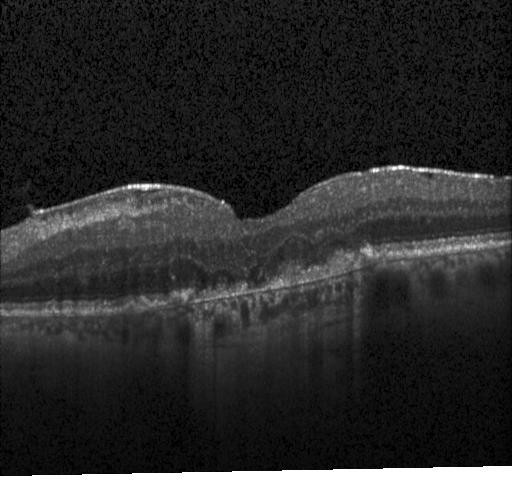 Retinal OCT B-scan
Impression: a choroidal neovascular membrane.